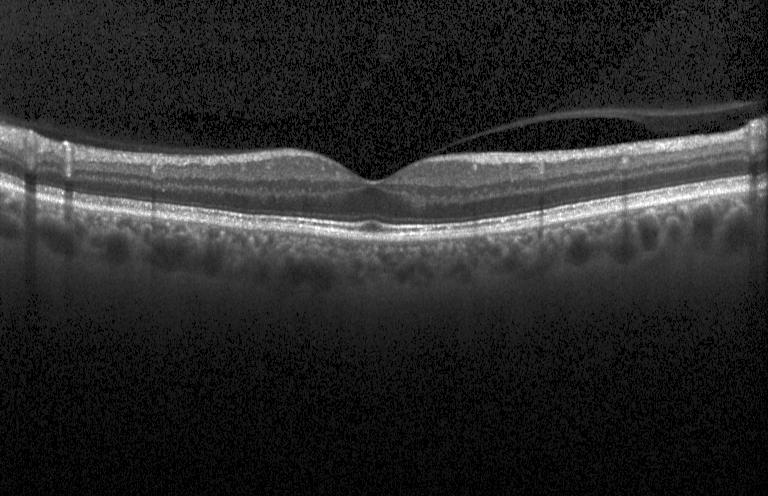 Spectral-domain OCT · macular scan · retinal OCT cross-section · acquired on a Heidelberg Spectralis. OCT finding: no CNV, DME, or drusen.